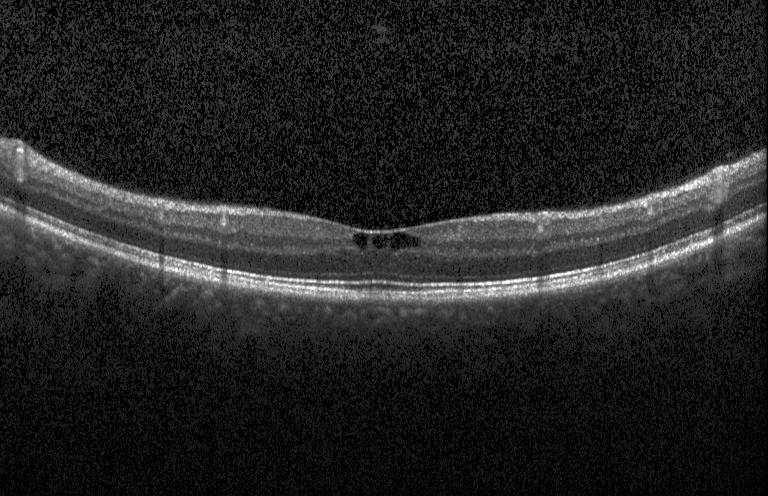
Impression: DME.